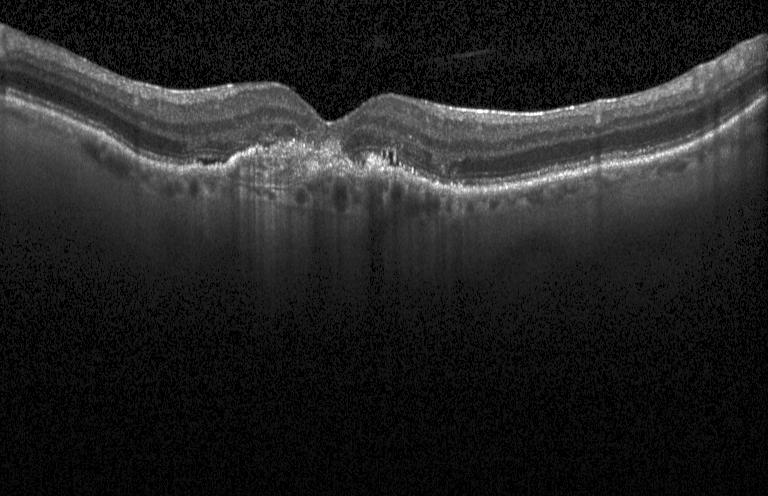

Impression: a choroidal neovascular membrane.